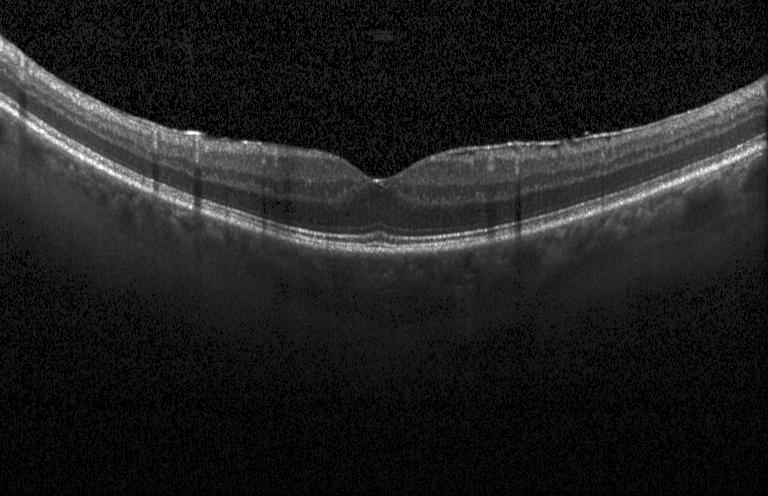

The scan shows no choroidal neovascularization, no diabetic macular edema, and no drusen.